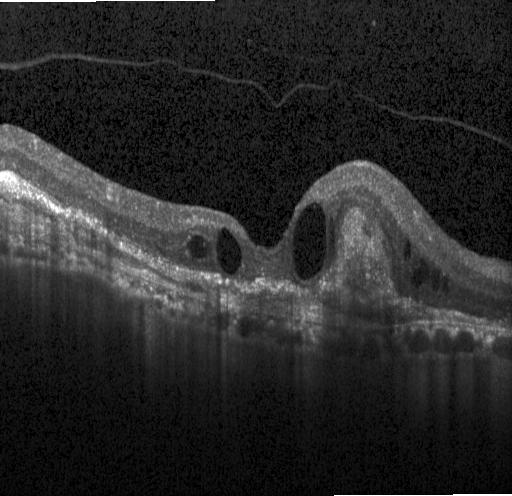

Horizontal scan through the fovea · retinal OCT B-scan · acquired on a Heidelberg Spectralis. Assessment: a choroidal neovascular membrane.